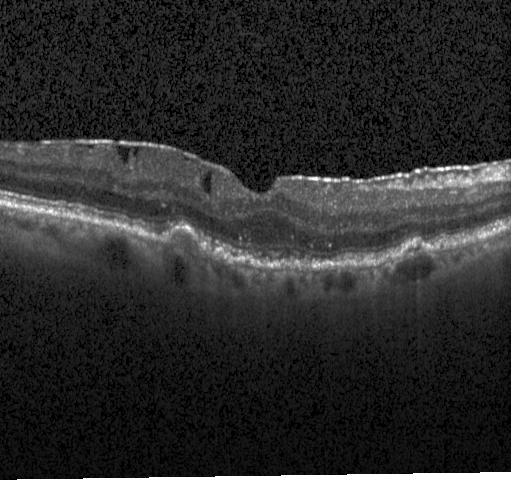

OCT line scan; spectral-domain OCT; Heidelberg Spectralis OCT system.
Finding: drusen.